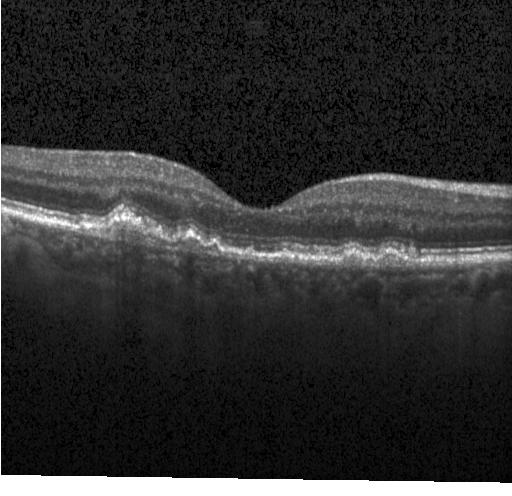
Horizontal scan through the fovea · OCT line scan — The scan shows choroidal neovascularization (CNV).